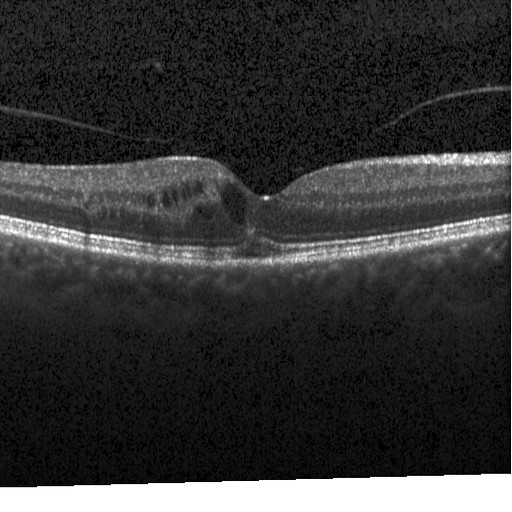

Impression: diabetic macular edema (DME).